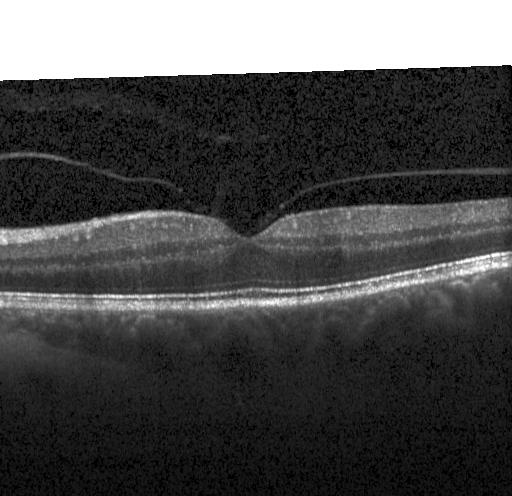 Retinal OCT cross-section showing neither choroidal neovascularization, diabetic macular edema, nor drusen.